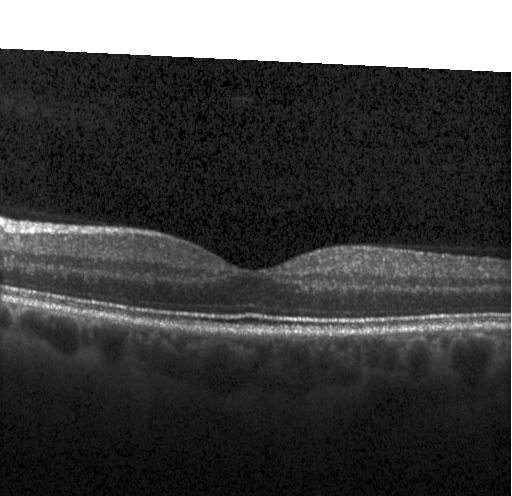
Diagnosis: neither choroidal neovascularization, diabetic macular edema, nor drusen.